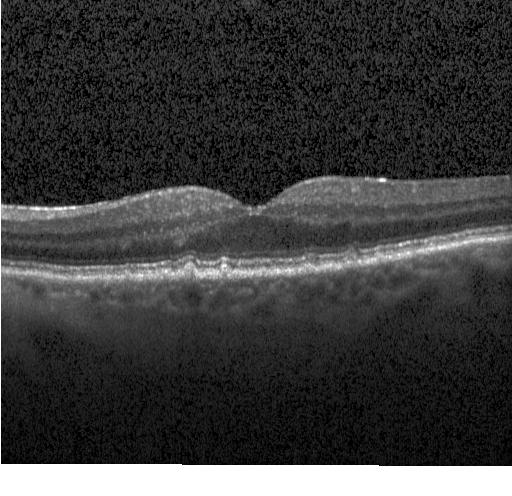 Macular scan; OCT line scan — Diagnosis: sub-RPE drusenoid deposits.